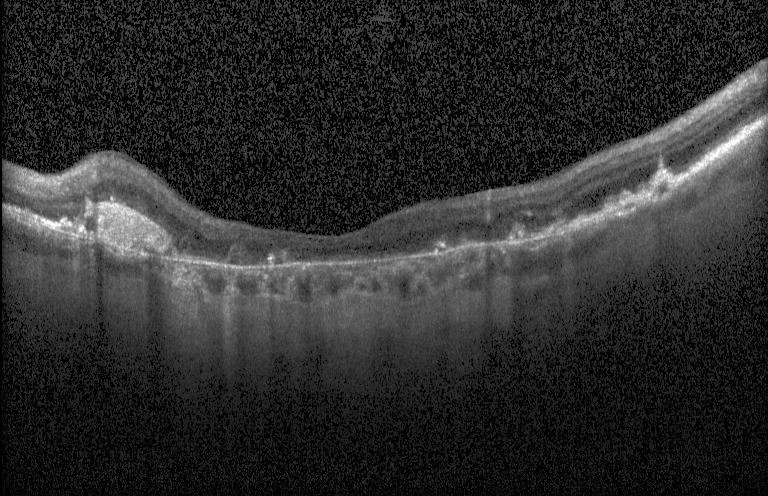
Impression: a choroidal neovascular membrane.